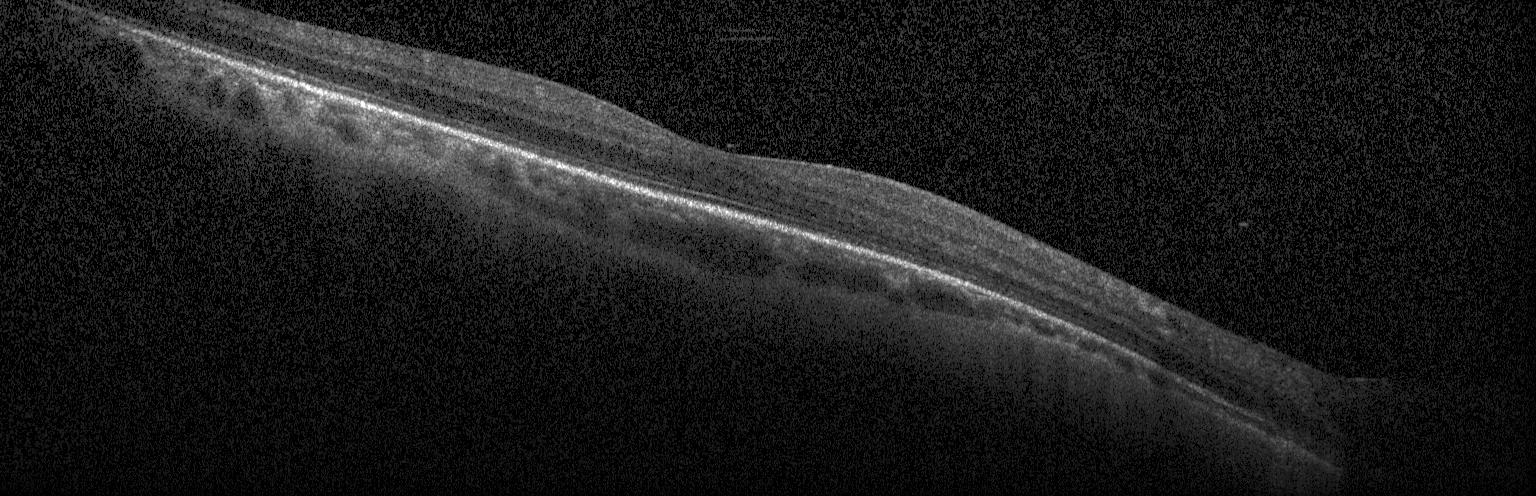
Spectral-domain optical coherence tomography; horizontal scan through the fovea; Heidelberg Spectralis; optical coherence tomography B-scan. Diagnosis: neither choroidal neovascularization, diabetic macular edema, nor drusen.